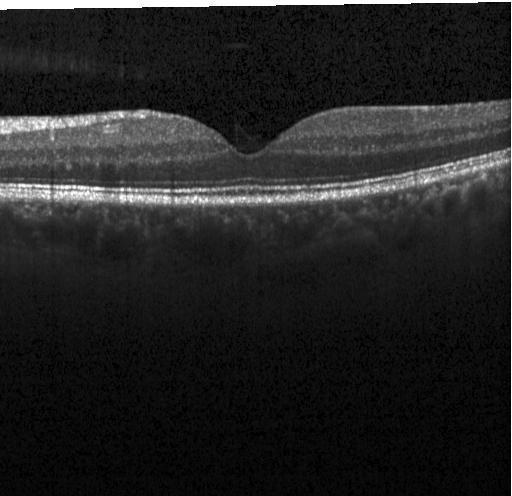
Diagnosis: no CNV, no DME, and no drusen.